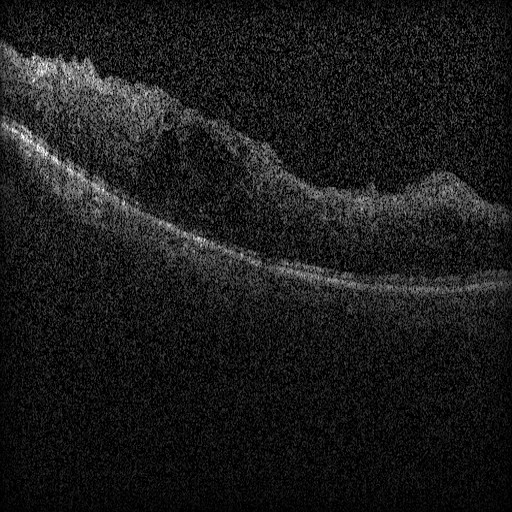
Macular OCT: diabetic macular edema.